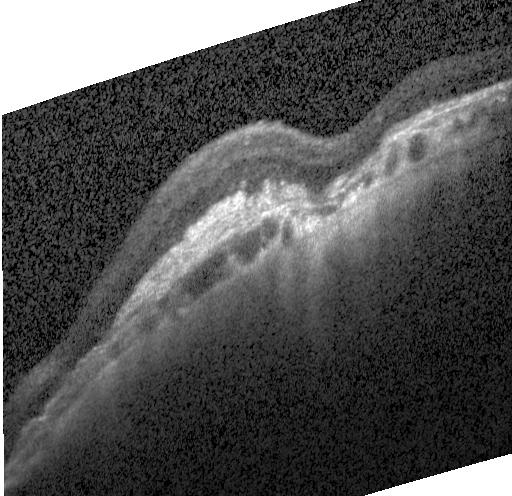

OCT scan showing a choroidal neovascular membrane.